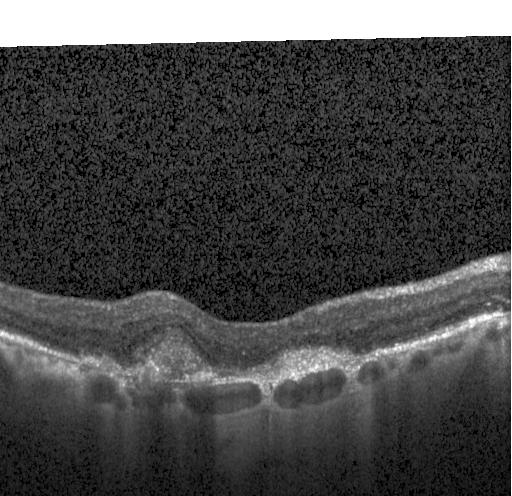
Spectral-domain OCT B-scan: a choroidal neovascular membrane.